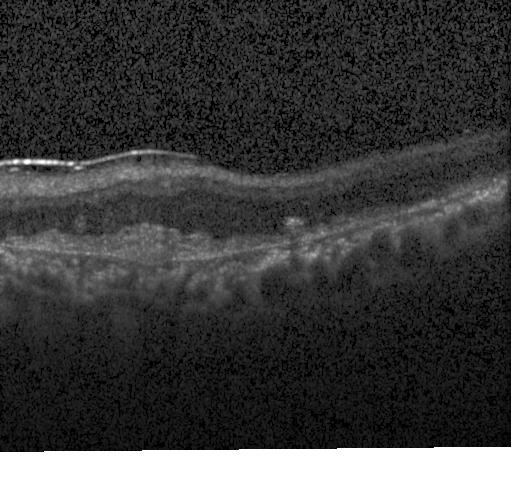
Diagnosis: a choroidal neovascular membrane.